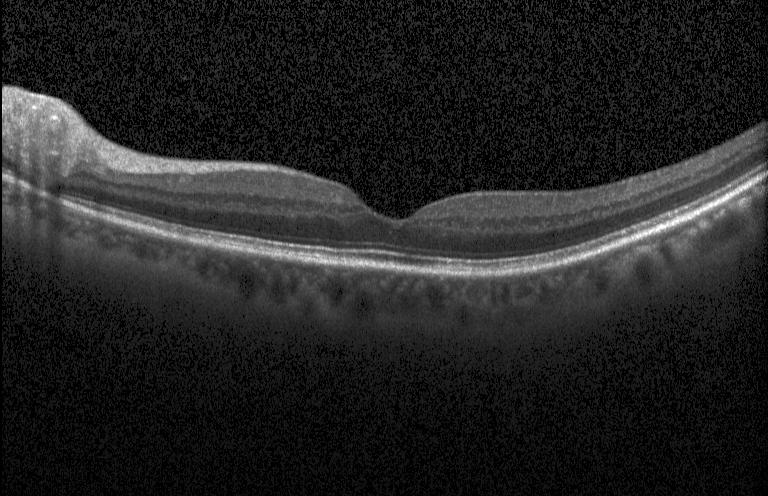

OCT B-scan · Heidelberg Spectralis OCT system · macular scan
No choroidal neovascularization, no diabetic macular edema, and no drusen.